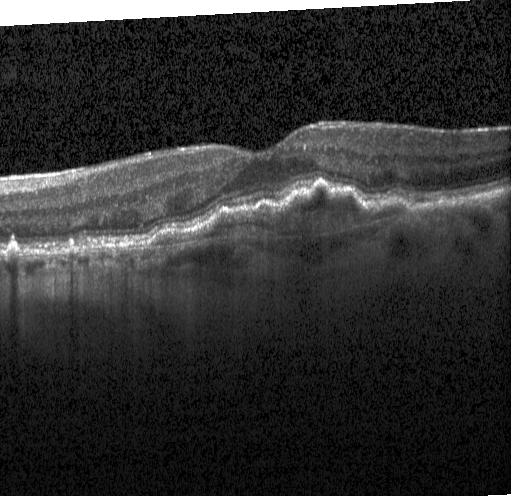

OCT line scan · SD-OCT · acquired on a Heidelberg Spectralis · centered on the fovea
Choroidal neovascularization.